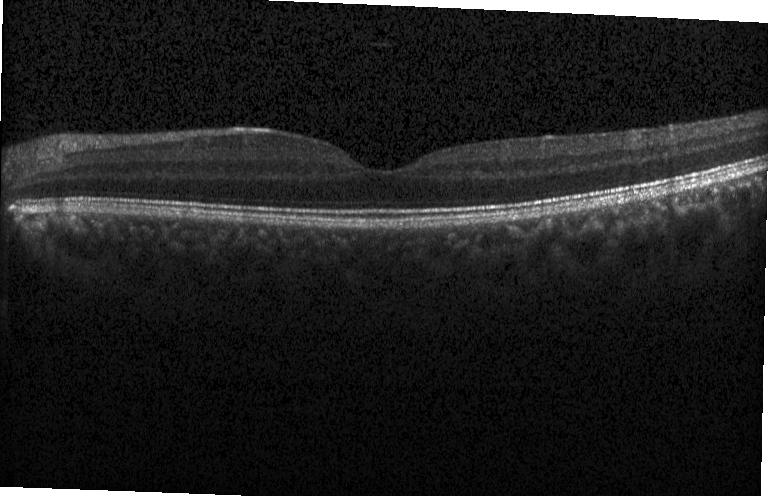
SD-OCT, retinal OCT cross-section, through the macula. The scan shows no choroidal neovascularization, no diabetic macular edema, and no drusen.